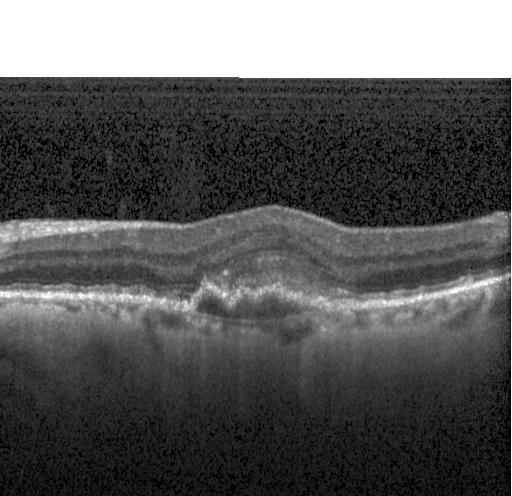
Macular OCT: a choroidal neovascular membrane.